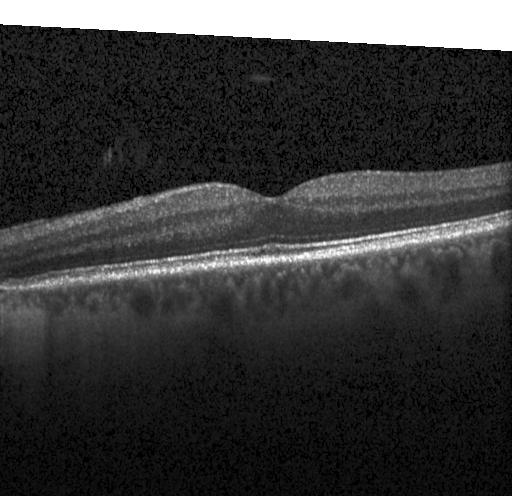

Macular OCT demonstrating no choroidal neovascularization, diabetic macular edema, or drusen.